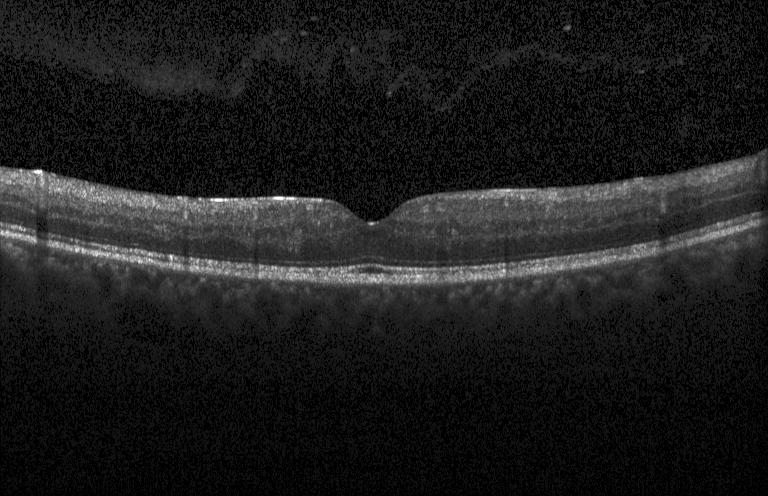

OCT line scan — Assessment: no choroidal neovascularization, diabetic macular edema, or drusen.